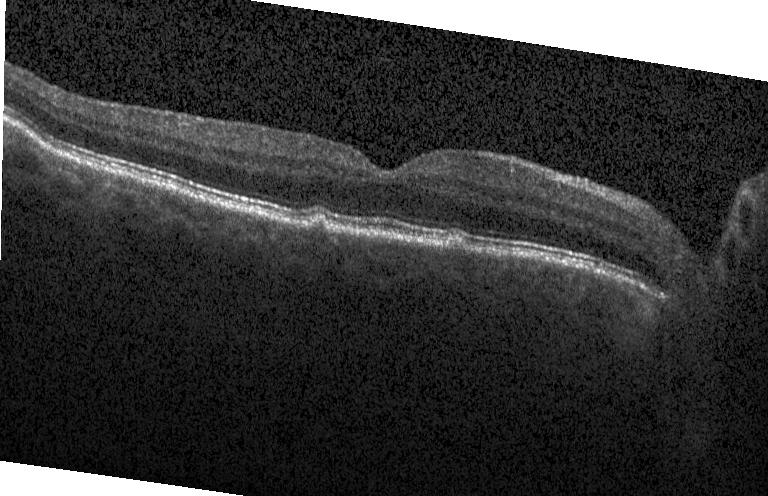 Heidelberg Spectralis OCT system · spectral-domain optical coherence tomography · optical coherence tomography B-scan
Finding: sub-RPE drusenoid deposits.